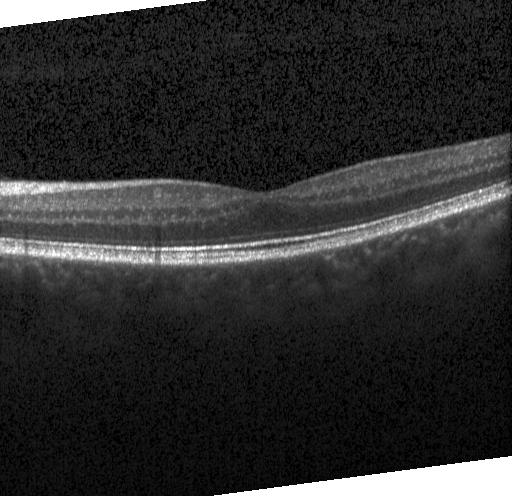
Retinal OCT B-scan
The scan shows no CNV, DME, or drusen.